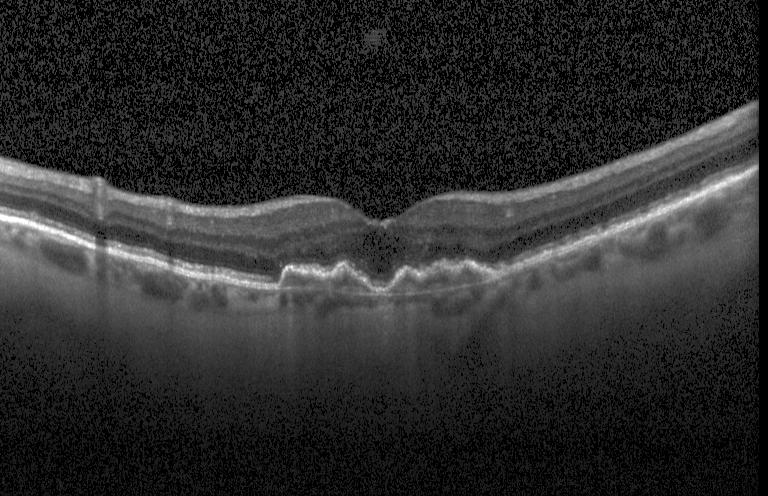

OCT B-scan showing a choroidal neovascular membrane.